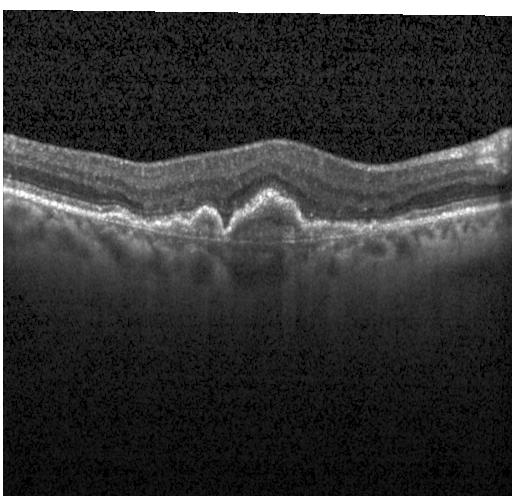 Through the macula; optical coherence tomography scan; spectral-domain optical coherence tomography. OCT finding: choroidal neovascularization (CNV).